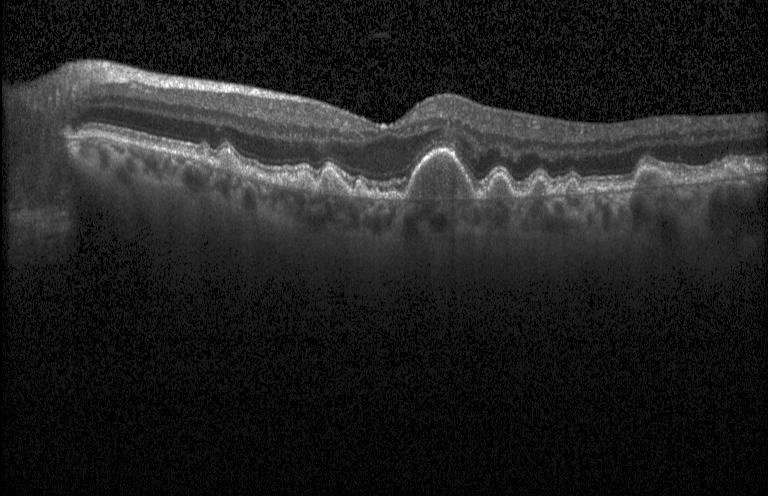 OCT B-scan, spectral-domain OCT — Impression: sub-RPE drusenoid deposits.